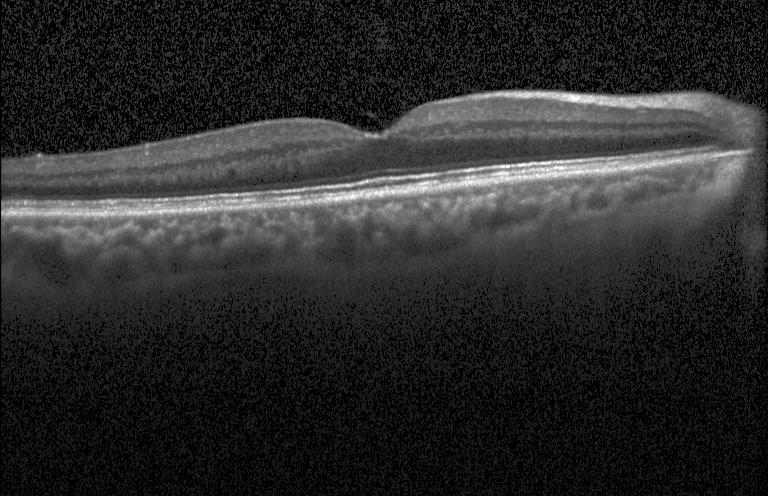 Through the macula, acquired on a Heidelberg Spectralis, retinal OCT cross-section, spectral-domain OCT
Finding: no CNV, no DME, and no drusen.